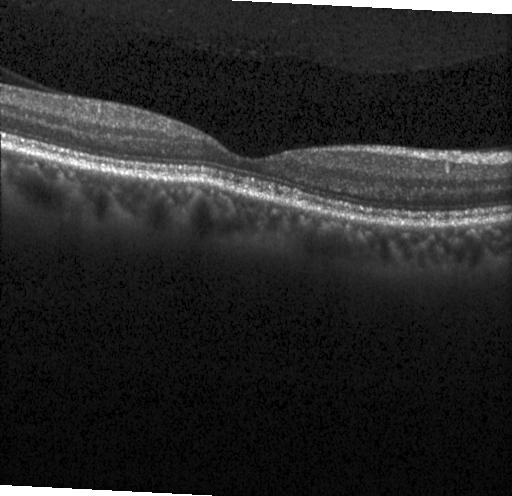

Heidelberg Spectralis; OCT line scan
Finding: no evidence of CNV, DME, or drusen.